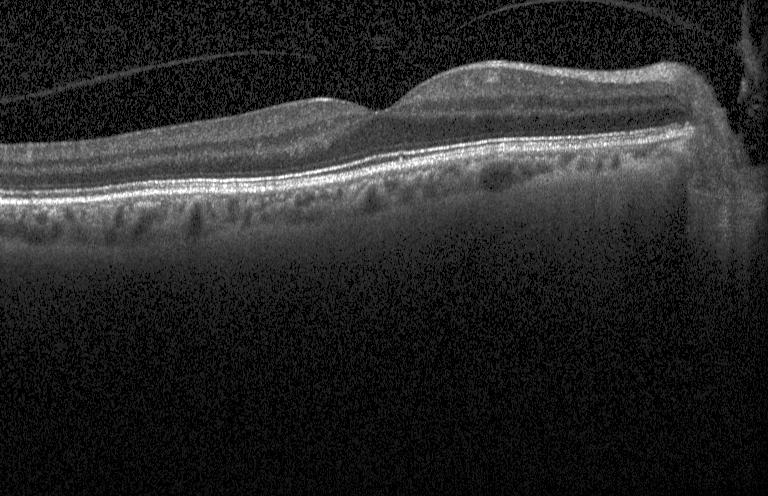
OCT line scan. SD-OCT. Fovea-centered. Heidelberg Spectralis. No CNV, no DME, and no drusen.